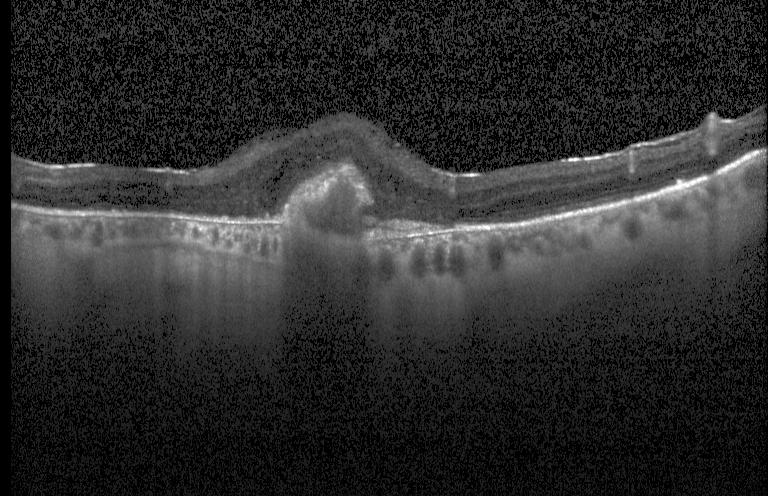
Fovea-centered · SD-OCT · OCT line scan · instrument: Heidelberg Spectralis — The scan shows choroidal neovascularization (CNV).